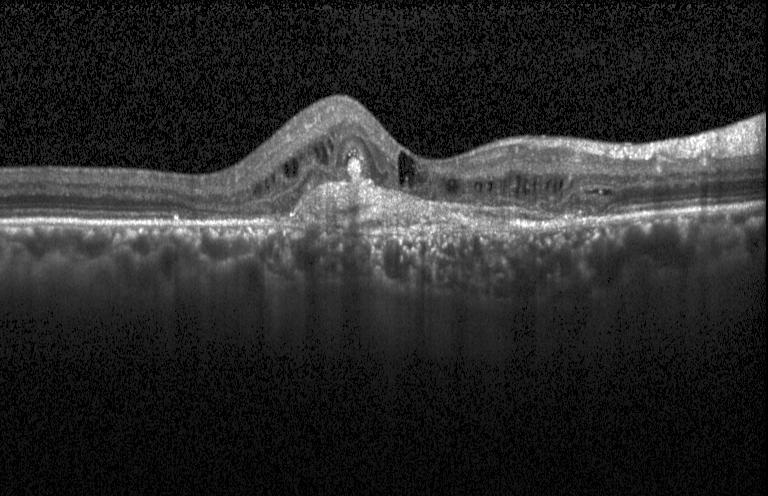

Macular OCT: CNV.